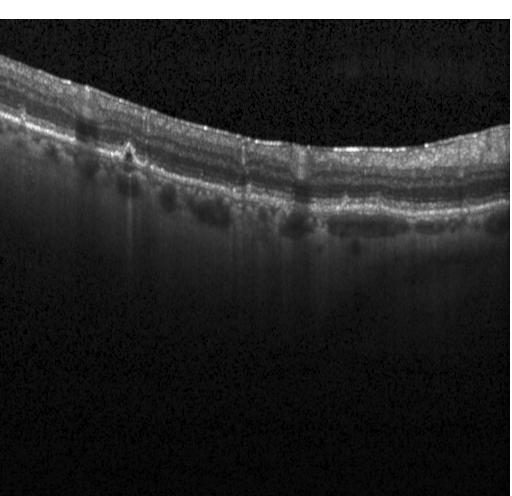

Heidelberg Spectralis OCT system. OCT B-scan. Spectral-domain optical coherence tomography. Fovea-centered — Impression: a choroidal neovascular membrane.